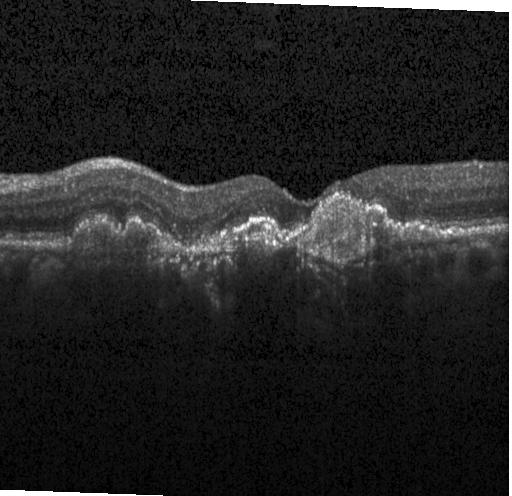 Macular scan. Retinal OCT B-scan
Diagnosis: a choroidal neovascular membrane.